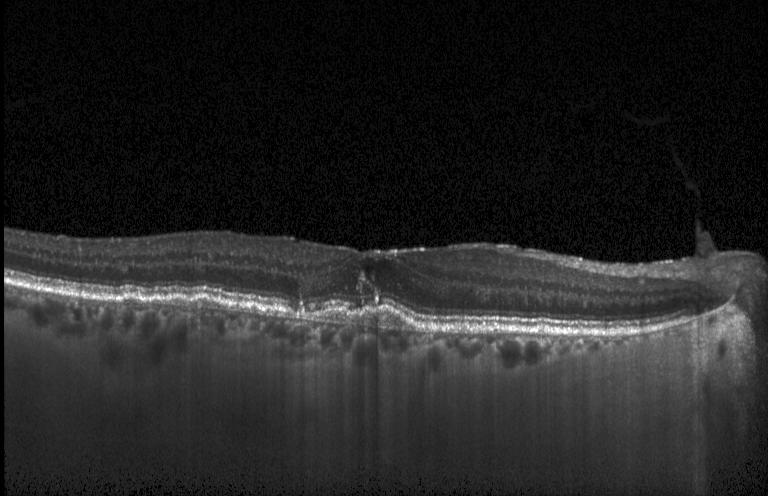
Assessment: choroidal neovascularization.